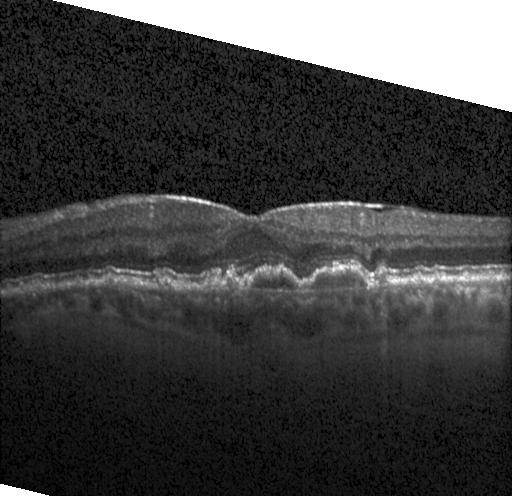
Heidelberg Spectralis OCT system. Retinal OCT cross-section. Fovea-centered. SD-OCT. Drusen.